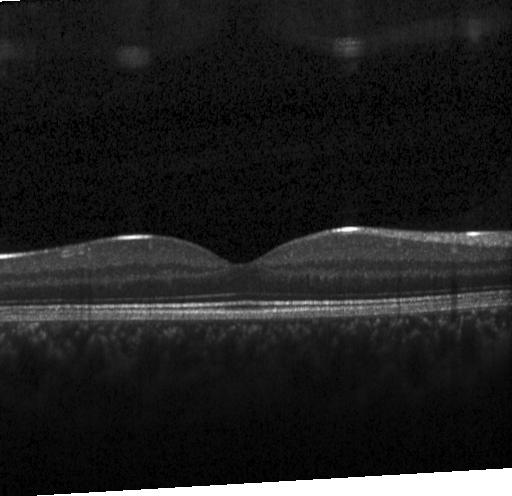
OCT line scan — Diagnosis: no choroidal neovascularization, no diabetic macular edema, and no drusen.